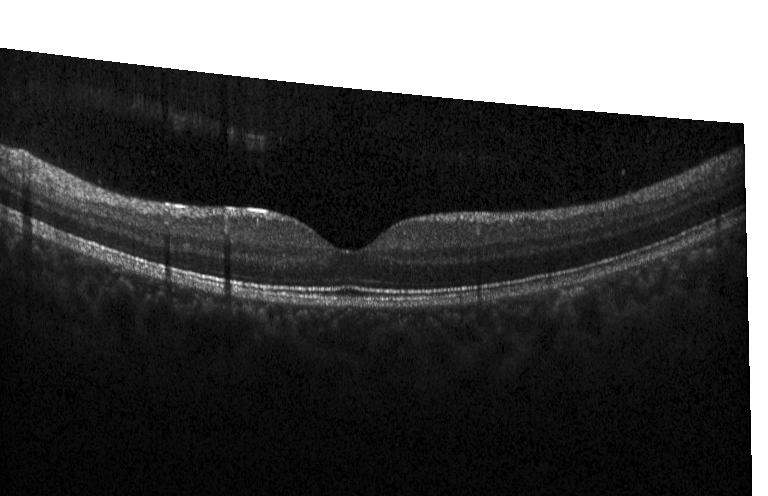
Heidelberg Spectralis, SD-OCT, optical coherence tomography B-scan, fovea-centered. Dx: no evidence of choroidal neovascularization, diabetic macular edema, or drusen.